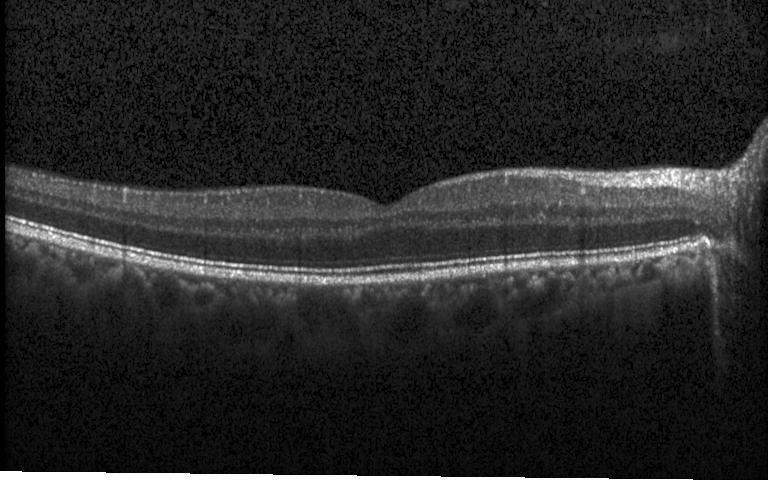 Retinal OCT cross-section
Diagnosis: no choroidal neovascularization, diabetic macular edema, or drusen.